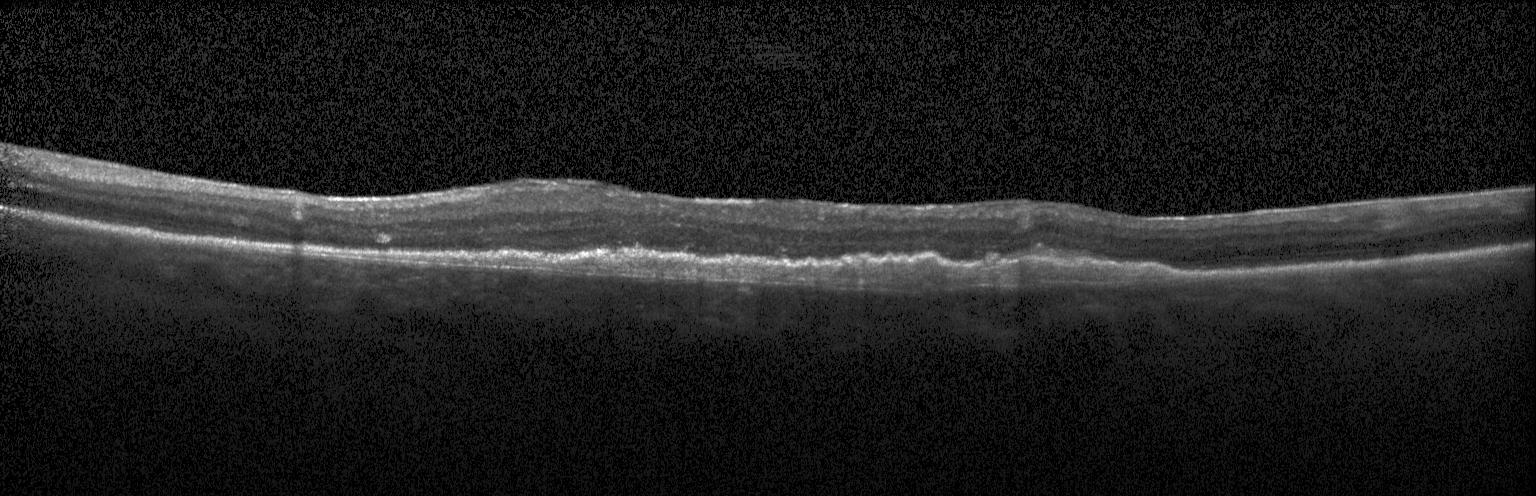

Optical coherence tomography B-scan.
Dx: CNV.